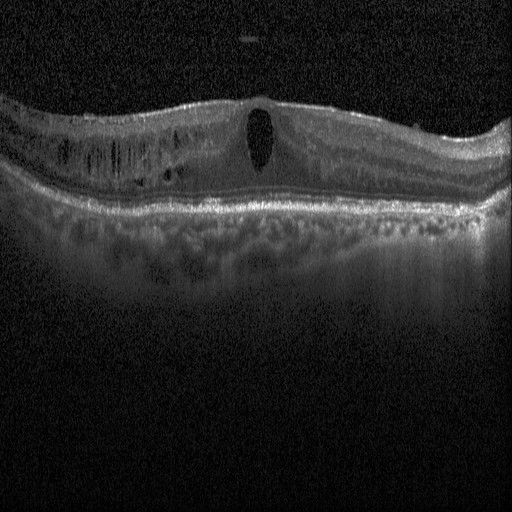

Optical coherence tomography scan · acquired on a Heidelberg Spectralis · SD-OCT. Macular OCT: DME.